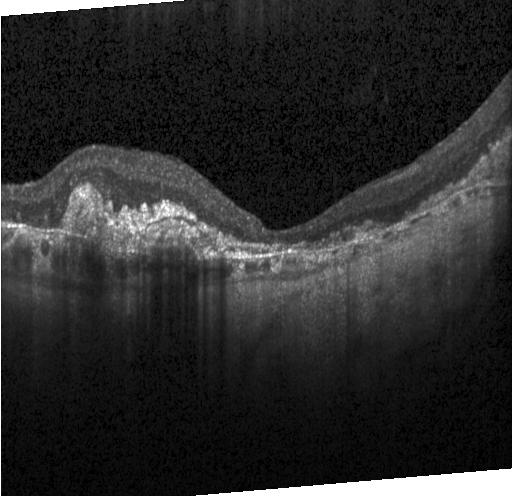

Acquired on a Heidelberg Spectralis, OCT line scan, macular scan
Macular OCT: a choroidal neovascular membrane.